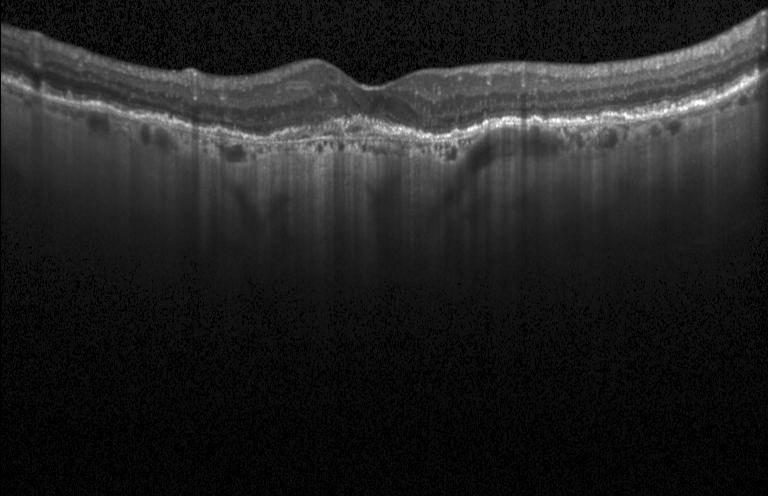
OCT B-scan. This B-scan demonstrates CNV.